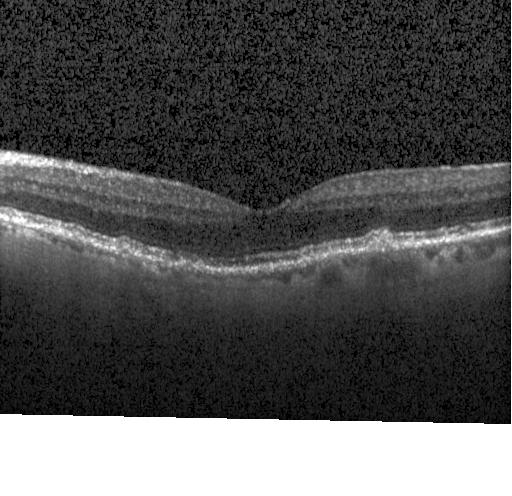 Spectral-domain OCT B-scan: drusen.